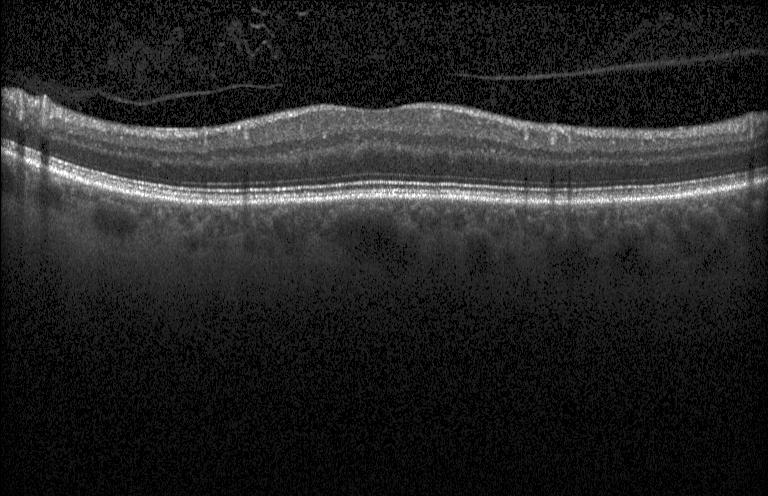
Fovea-centered; OCT B-scan; instrument: Heidelberg Spectralis; SD-OCT.
Finding: neither choroidal neovascularization, diabetic macular edema, nor drusen.